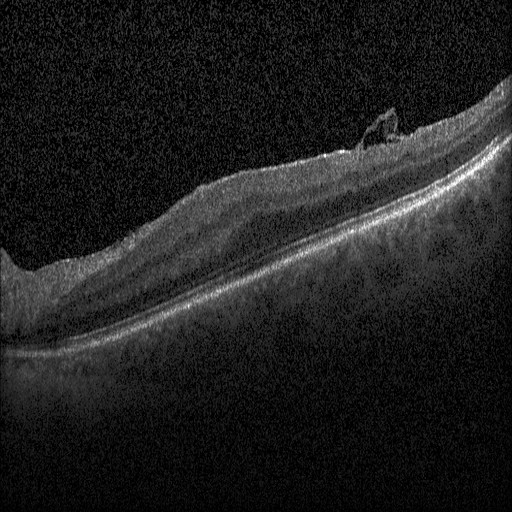 Through the macula, acquired on a Heidelberg Spectralis, SD-OCT, retinal OCT B-scan. Dx: diabetic macular edema (DME).